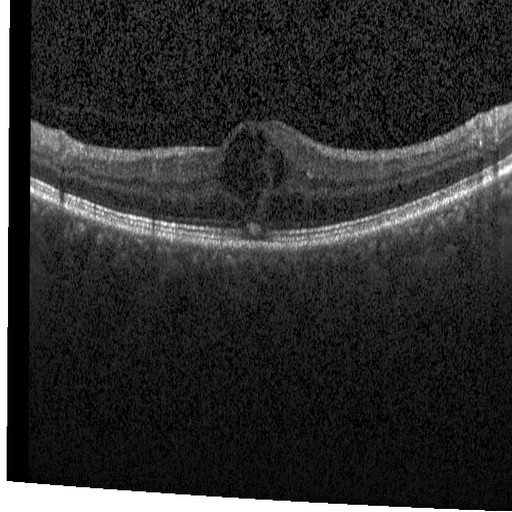
Impression: diabetic macular edema.